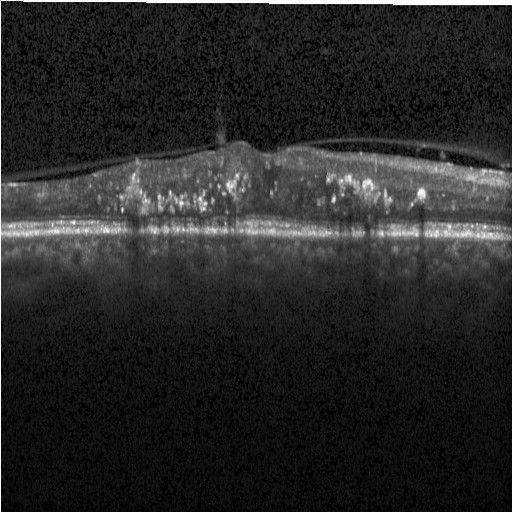
Finding: diabetic macular edema.